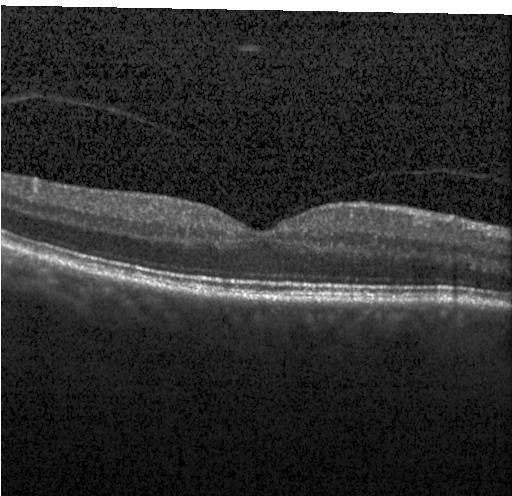

Optical coherence tomography B-scan. Spectral-domain optical coherence tomography. OCT finding: neither choroidal neovascularization, diabetic macular edema, nor drusen.